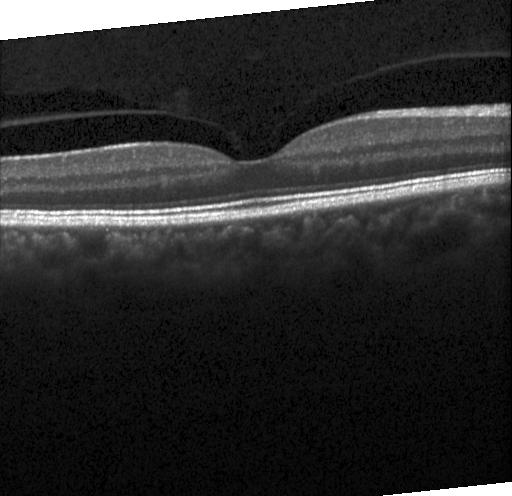
Acquired on a Heidelberg Spectralis · retinal OCT B-scan — Impression: neither choroidal neovascularization, diabetic macular edema, nor drusen.